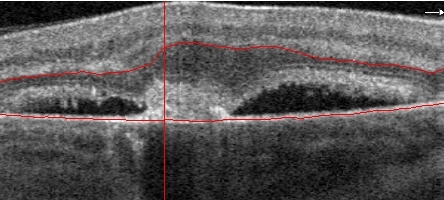
Optical coherence tomography B-scan — Diagnosis: age-related macular degeneration (AMD).